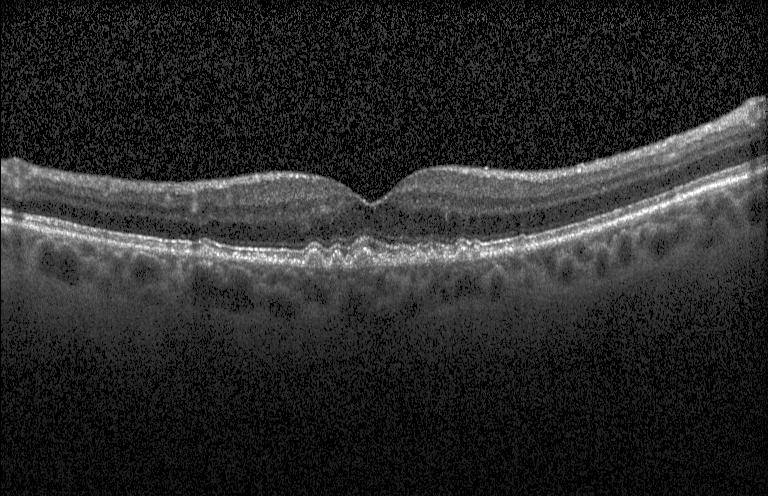 Acquired on a Heidelberg Spectralis. Macular scan. Retinal OCT cross-section
Macular OCT: sub-RPE drusenoid deposits.